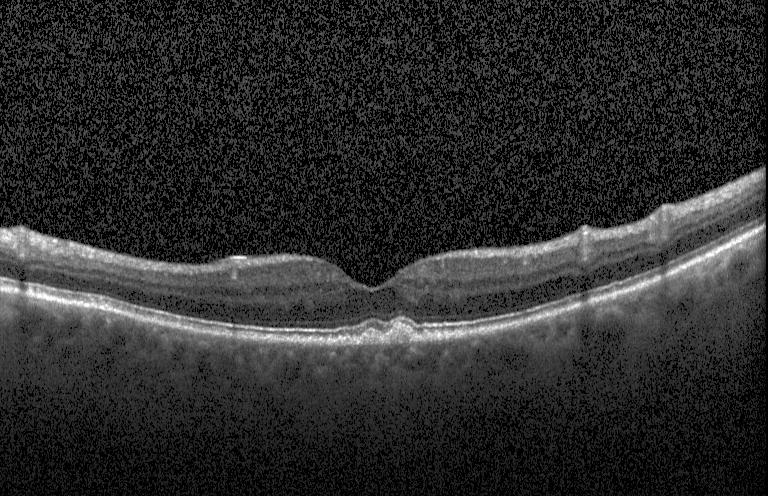 Fovea-centered. Retinal OCT cross-section. Heidelberg Spectralis. SD-OCT. Assessment: multiple drusen.